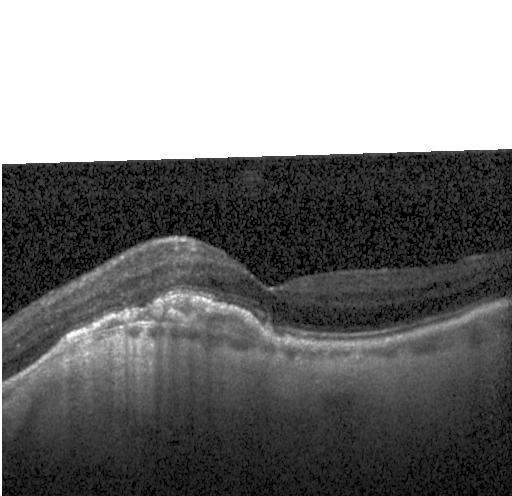
SD-OCT; OCT B-scan
Diagnosis: choroidal neovascularization.